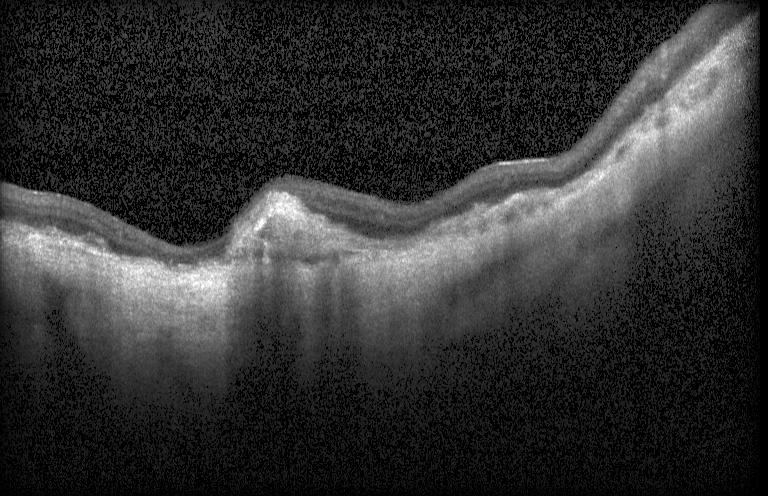

OCT scan showing CNV.